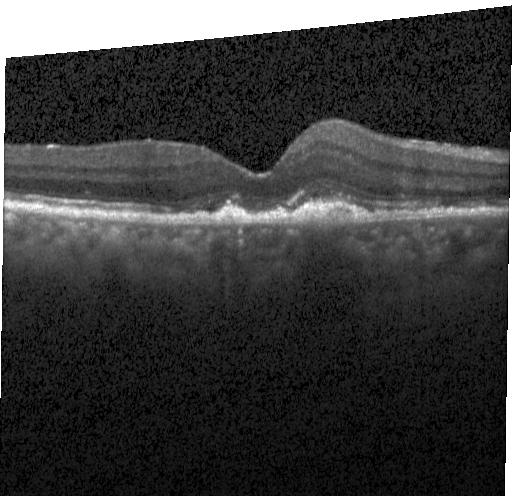

CNV.